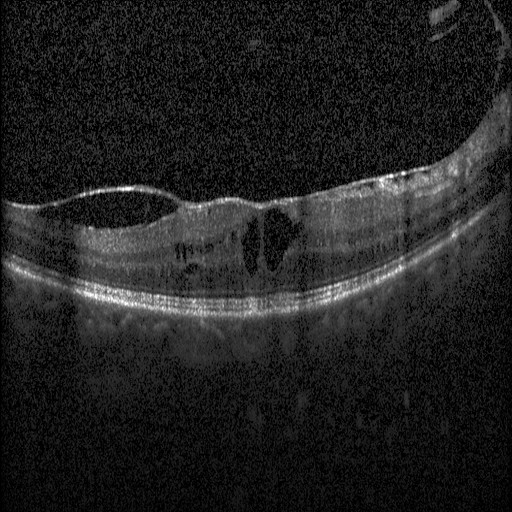
Centered on the fovea; retinal OCT B-scan — Impression: diabetic macular edema (DME).